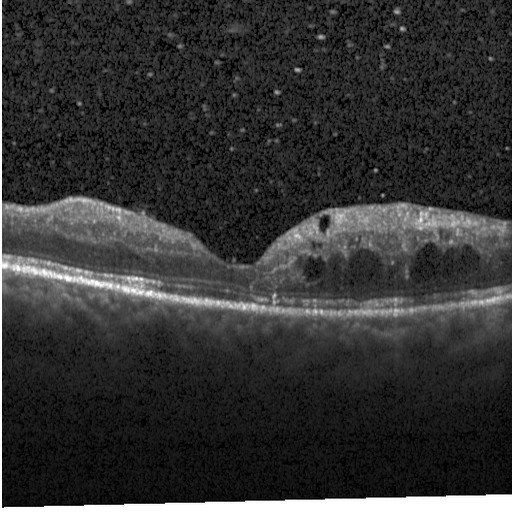
Impression: diabetic macular edema (DME).